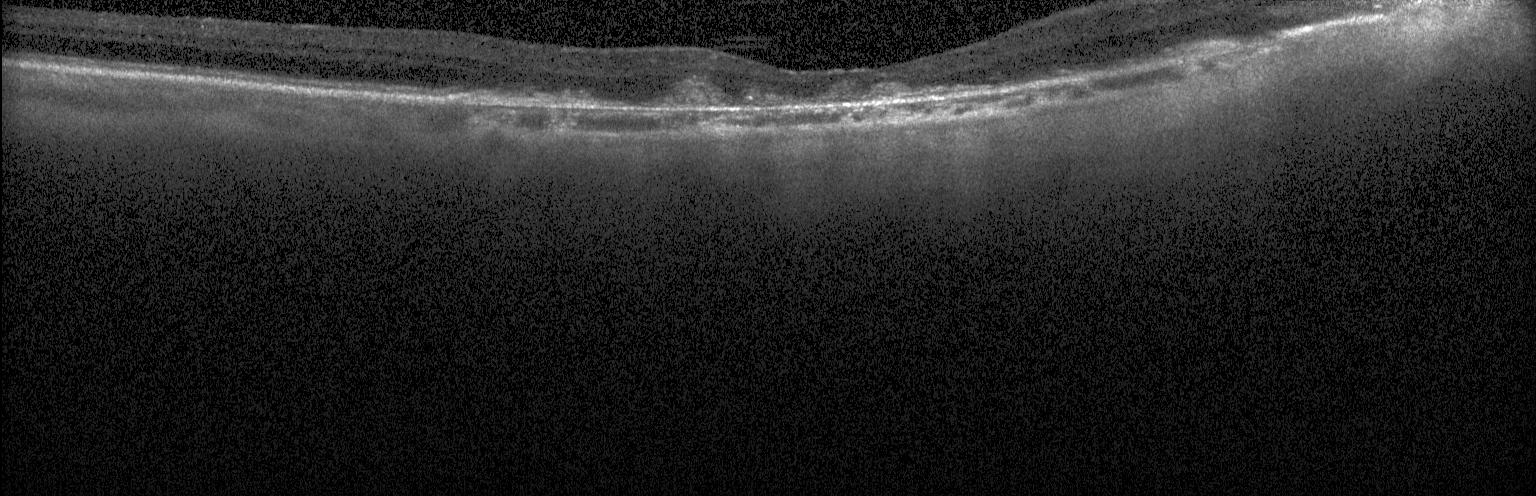

SD-OCT. Through the macula. Instrument: Heidelberg Spectralis. OCT B-scan
Assessment: a choroidal neovascular membrane.